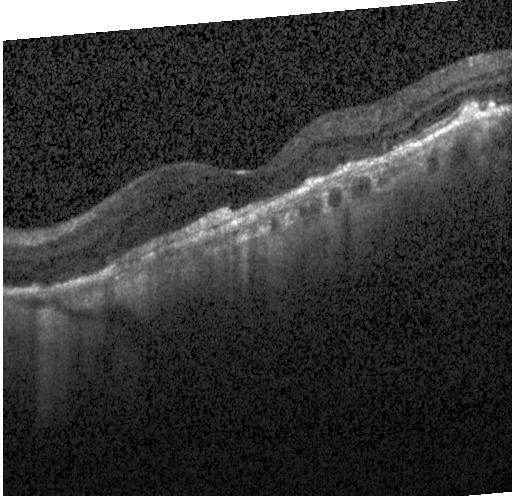

Retinal OCT B-scan — This B-scan demonstrates choroidal neovascularization.